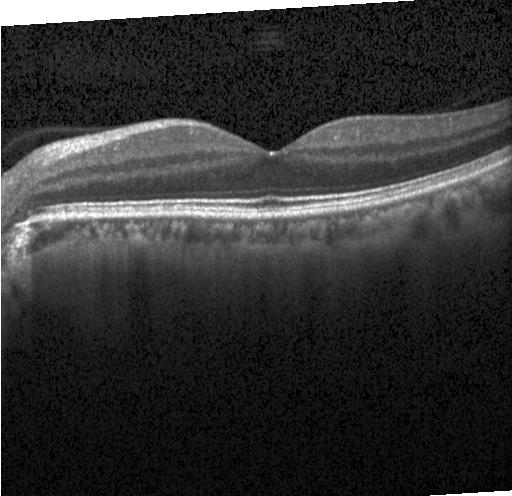
Heidelberg Spectralis OCT system; OCT B-scan; macular scan; spectral-domain OCT — OCT finding: neither choroidal neovascularization, diabetic macular edema, nor drusen.